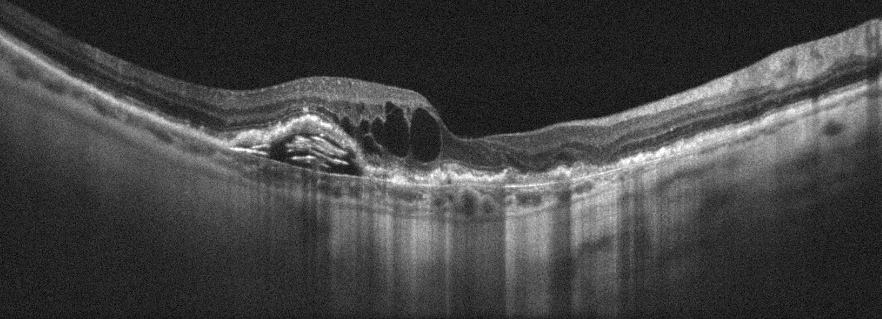 Oculus dexter. Retinal OCT cross-section. Diagnosis: AMD.